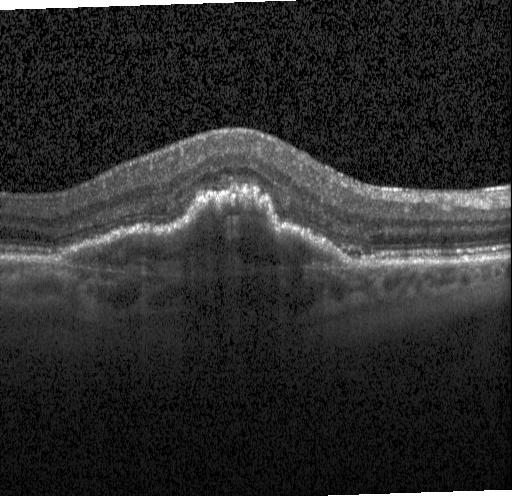 Finding: a choroidal neovascular membrane.